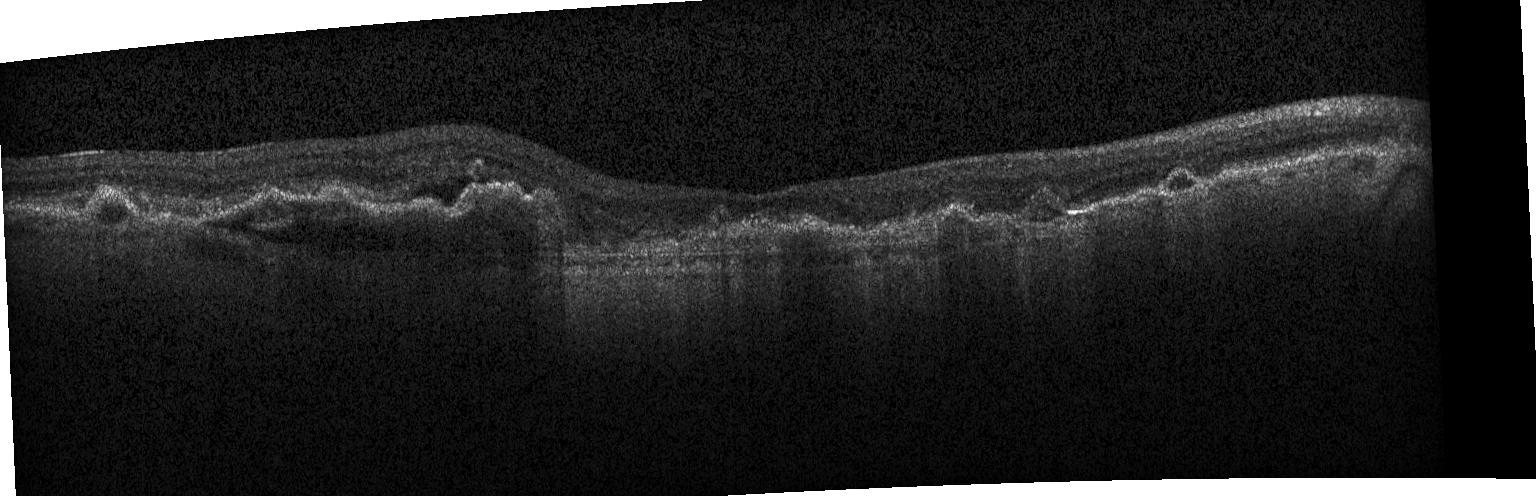 Heidelberg Spectralis OCT system · optical coherence tomography B-scan
A choroidal neovascular membrane.